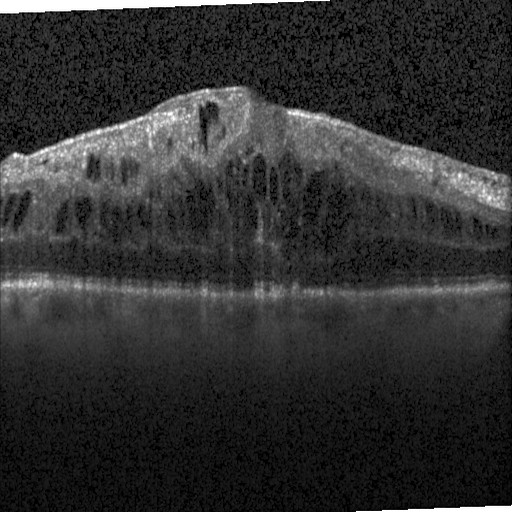 OCT B-scan. Diagnosis: diabetic macular edema (DME).